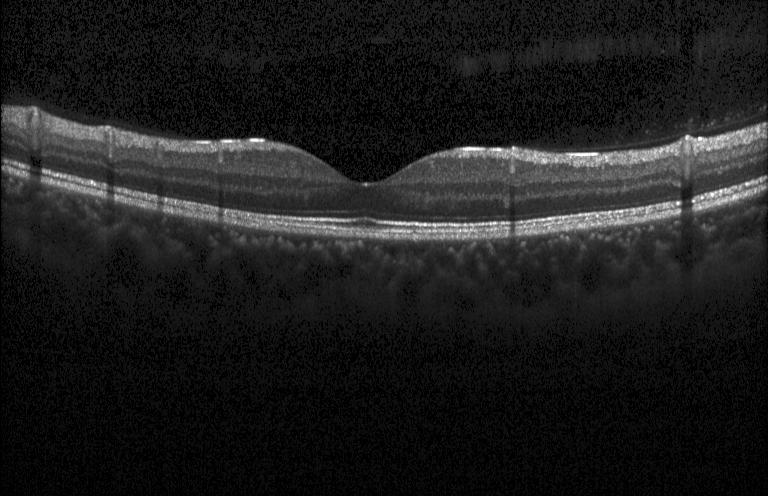
Retinal OCT B-scan — This B-scan demonstrates no evidence of CNV, DME, or drusen.